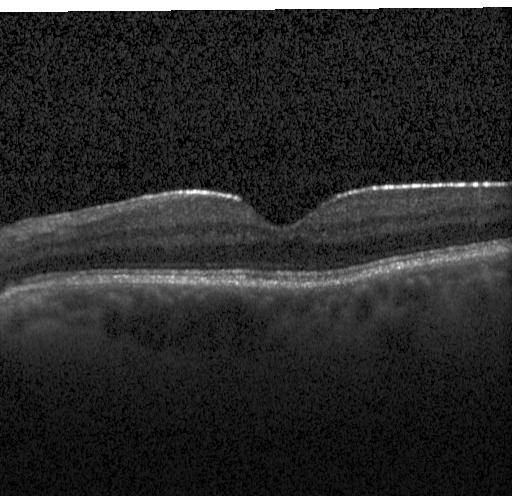
Dx: no CNV, DME, or drusen.